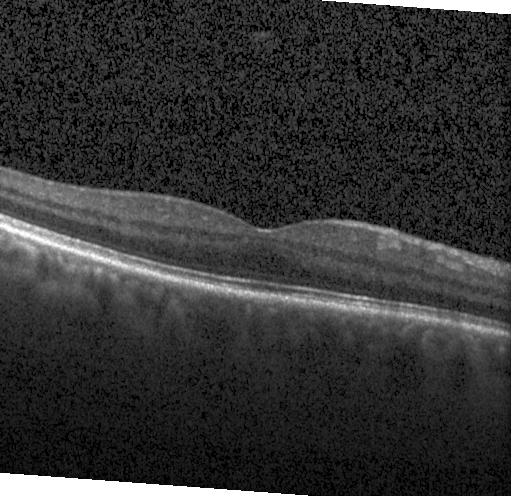 Acquired on a Heidelberg Spectralis. OCT B-scan. Fovea-centered. SD-OCT.
The scan shows neither choroidal neovascularization, diabetic macular edema, nor drusen.